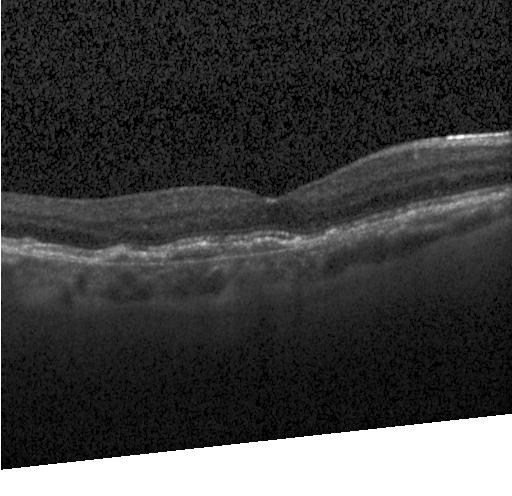
Optical coherence tomography B-scan. OCT finding: a choroidal neovascular membrane.